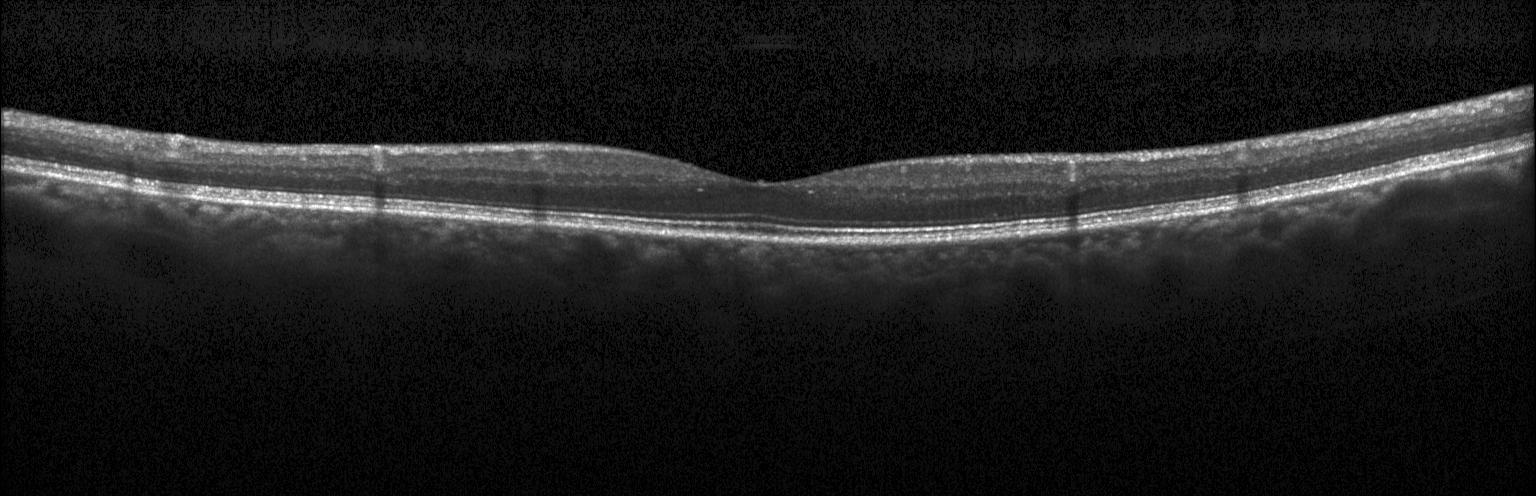

Retinal OCT B-scan. Heidelberg Spectralis. Spectral-domain optical coherence tomography
The scan shows no choroidal neovascularization, diabetic macular edema, or drusen.